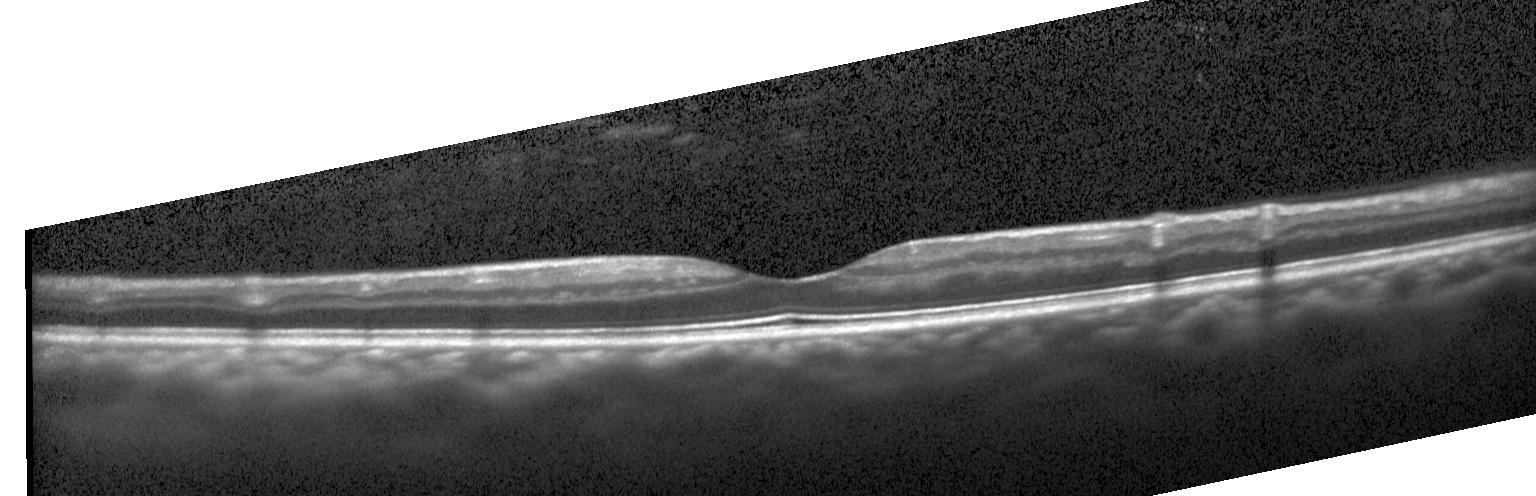

Spectral-domain OCT; optical coherence tomography scan
This B-scan demonstrates no evidence of choroidal neovascularization, diabetic macular edema, or drusen.